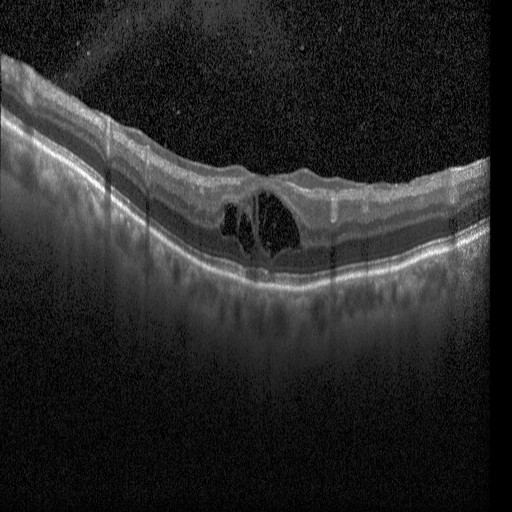 Macular OCT: DME.